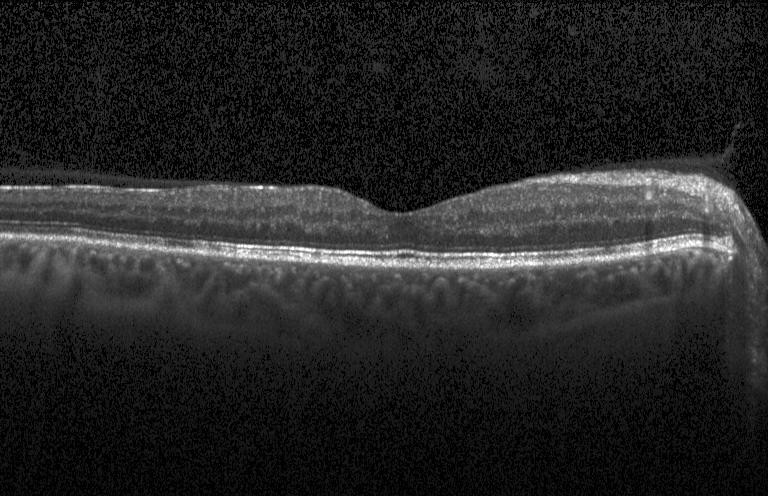
Heidelberg Spectralis OCT system, spectral-domain optical coherence tomography, OCT line scan
No evidence of choroidal neovascularization, diabetic macular edema, or drusen.